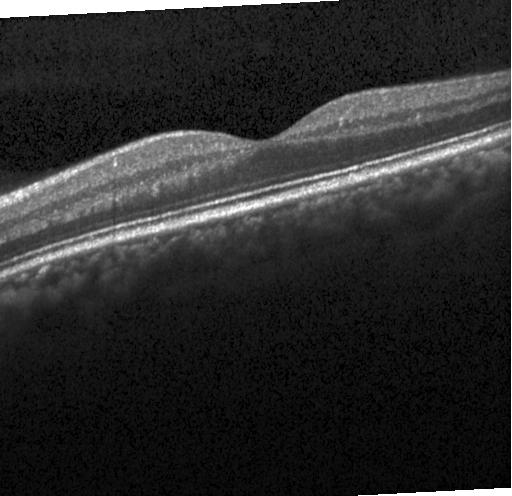 Impression: neither choroidal neovascularization, diabetic macular edema, nor drusen.